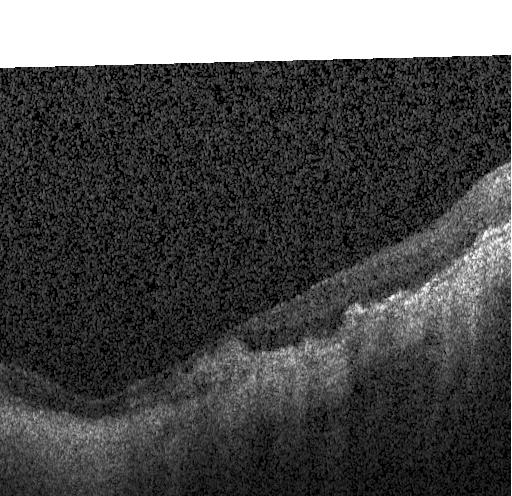

OCT finding: a choroidal neovascular membrane.